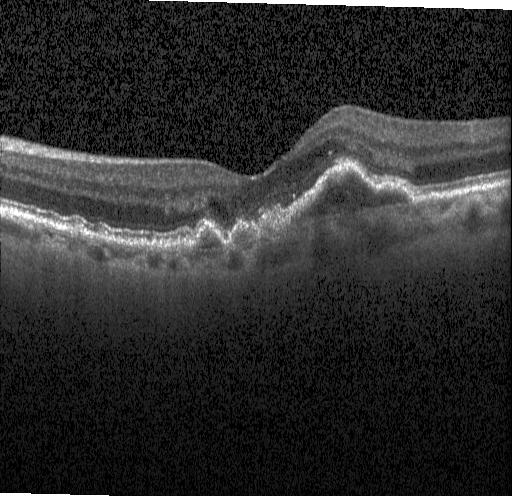 Retinal OCT B-scan
Finding: CNV.